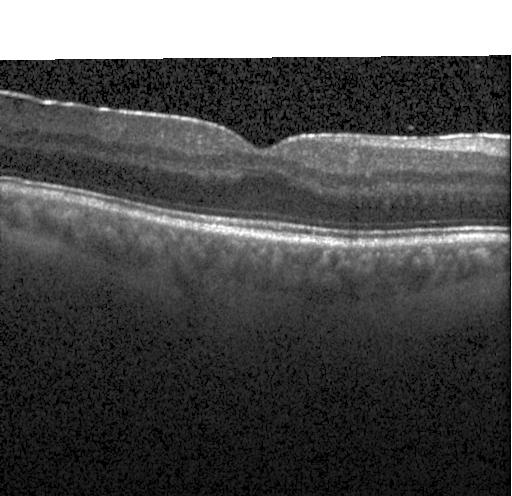
SD-OCT; Heidelberg Spectralis; retinal OCT cross-section
This B-scan demonstrates no evidence of choroidal neovascularization, diabetic macular edema, or drusen.